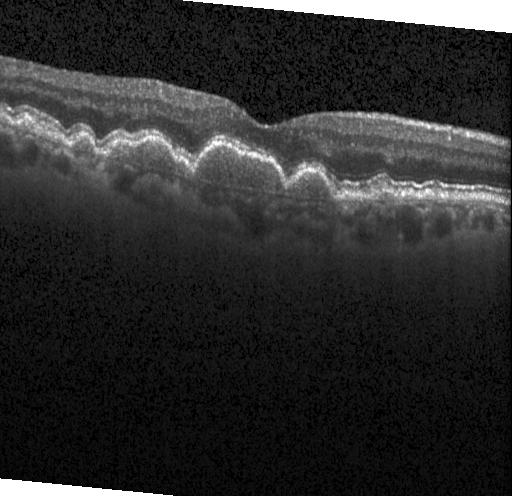

Spectral-domain OCT · centered on the fovea · retinal OCT B-scan
This B-scan demonstrates sub-RPE drusenoid deposits.